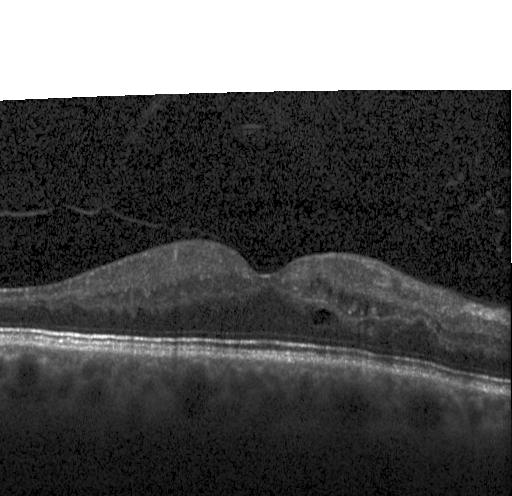
OCT B-scan · fovea-centered — The scan shows diabetic macular edema.